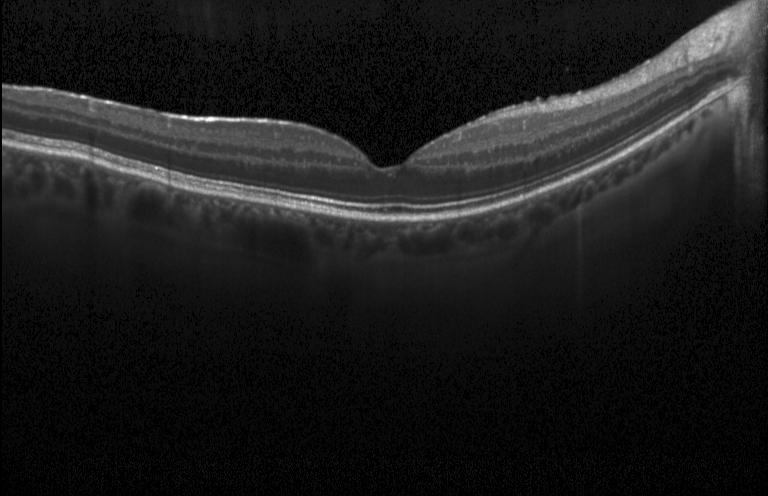

Impression: neither choroidal neovascularization, diabetic macular edema, nor drusen.